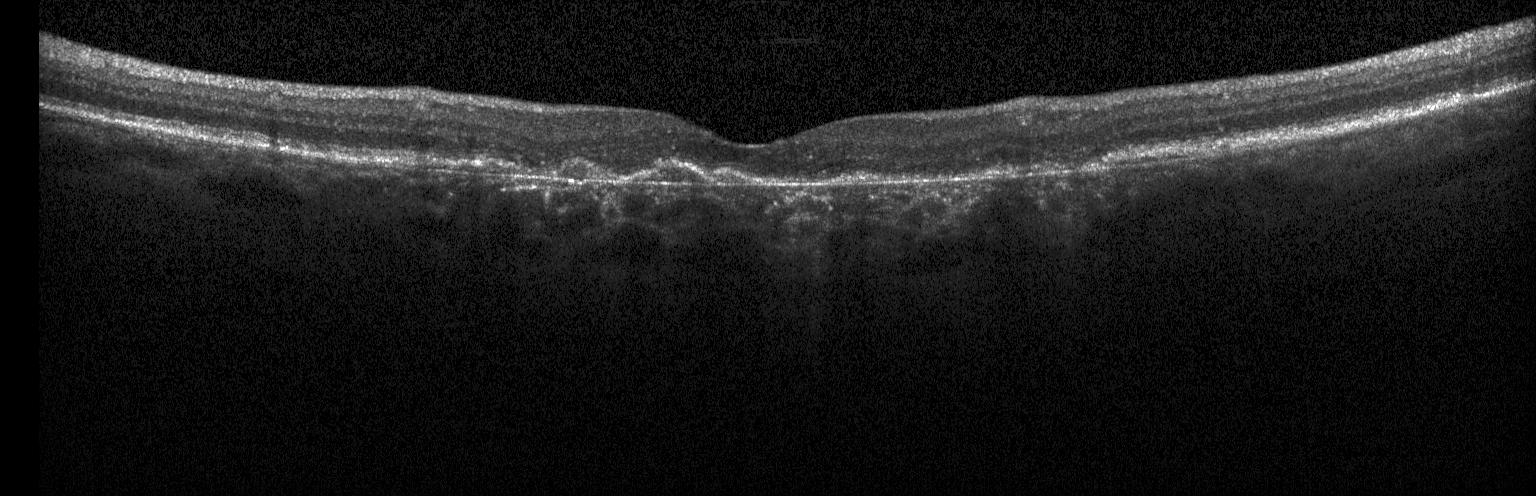

Spectral-domain OCT, optical coherence tomography scan
This B-scan demonstrates choroidal neovascularization.